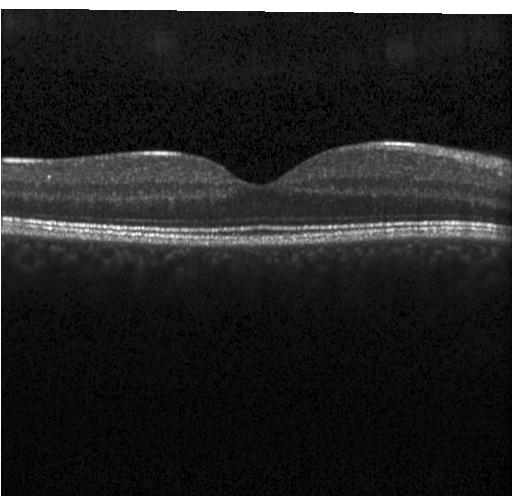

Dx: neither CNV, DME, nor drusen.